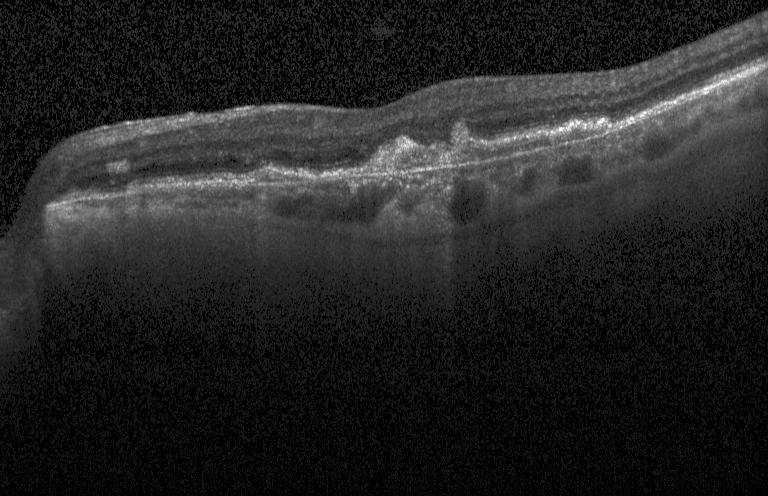
Through the macula · spectral-domain OCT · OCT B-scan. Finding: CNV.